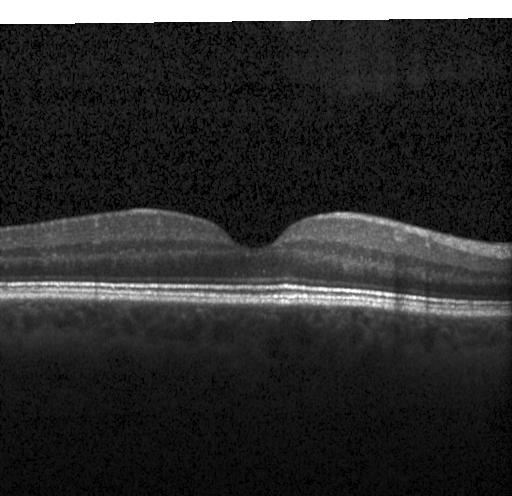

No evidence of choroidal neovascularization, diabetic macular edema, or drusen.